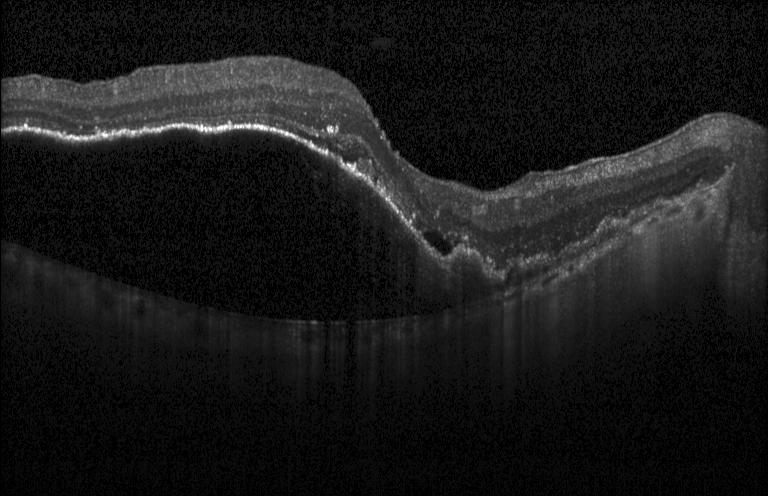
Fovea-centered, spectral-domain OCT, OCT line scan.
Macular OCT: a choroidal neovascular membrane.